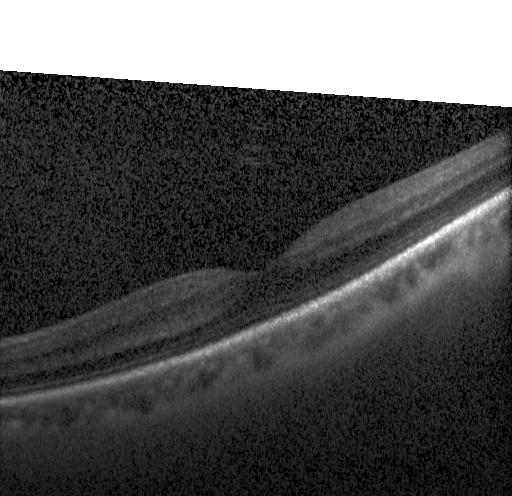 Heidelberg Spectralis, OCT line scan — Assessment: neither choroidal neovascularization, diabetic macular edema, nor drusen.